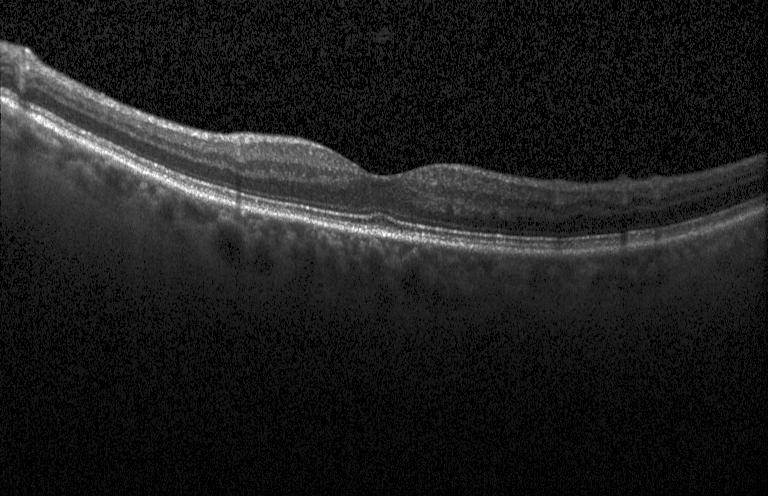
Spectral-domain OCT, optical coherence tomography B-scan.
Assessment: no choroidal neovascularization, no diabetic macular edema, and no drusen.